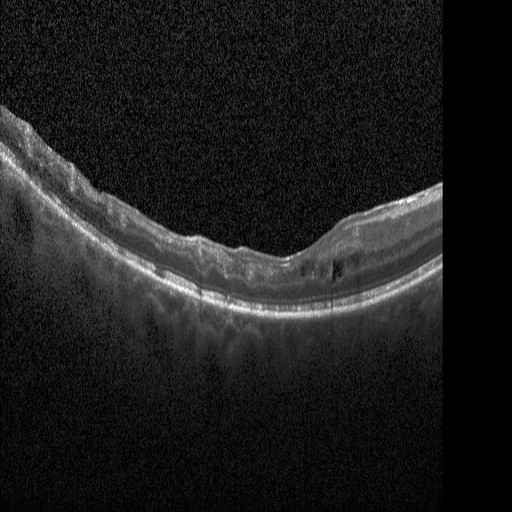
Retinal OCT cross-section; macular scan; acquired on a Heidelberg Spectralis — Assessment: diabetic macular edema.